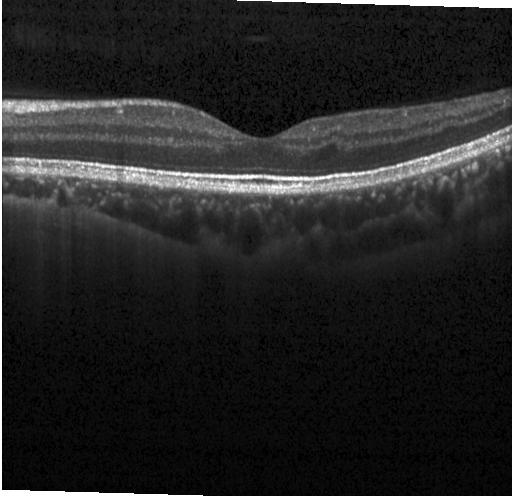 Centered on the fovea · OCT B-scan · Heidelberg Spectralis · spectral-domain OCT. Diagnosis: no choroidal neovascularization, no diabetic macular edema, and no drusen.